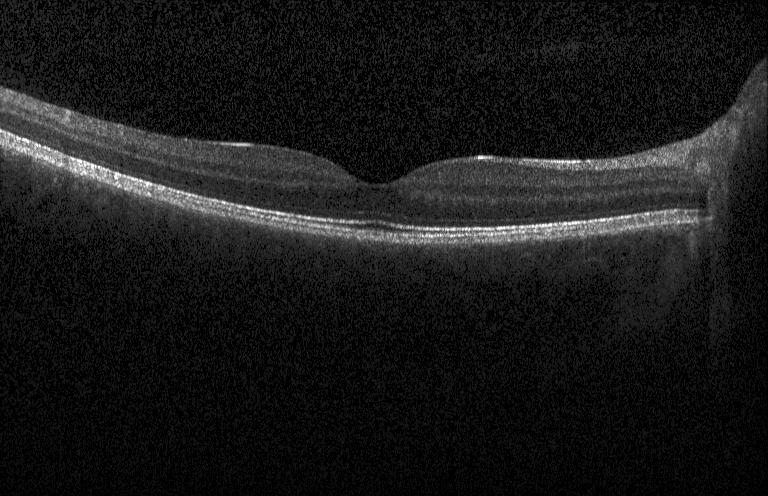

OCT line scan — Finding: no evidence of CNV, DME, or drusen.